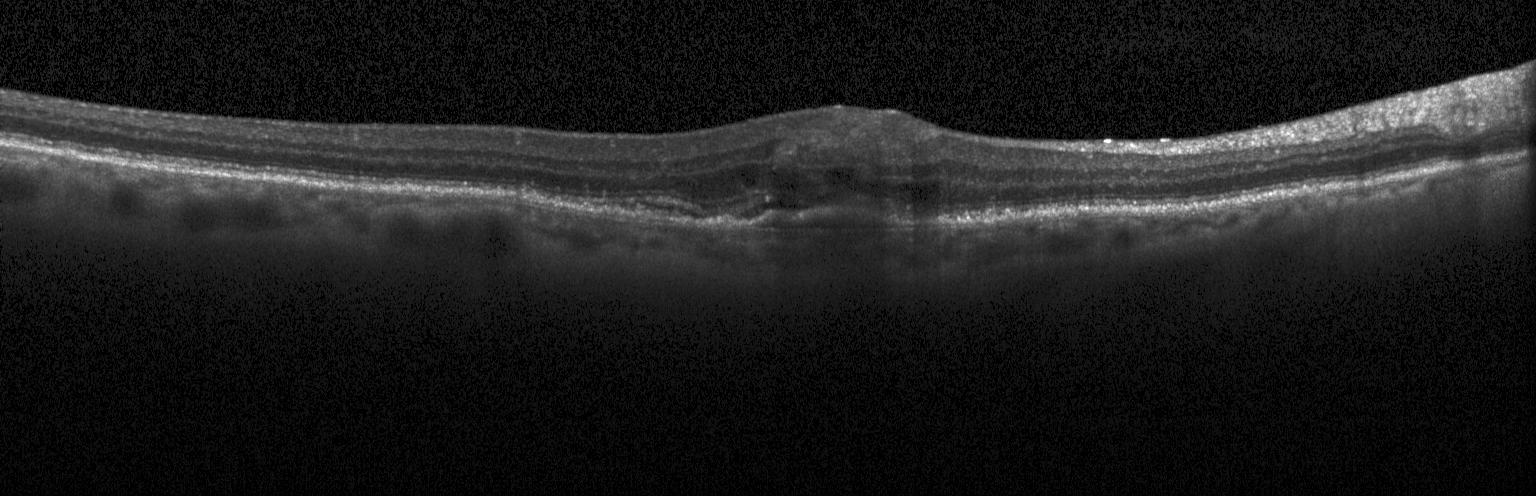
OCT line scan; centered on the fovea; Heidelberg Spectralis.
Dx: a choroidal neovascular membrane.